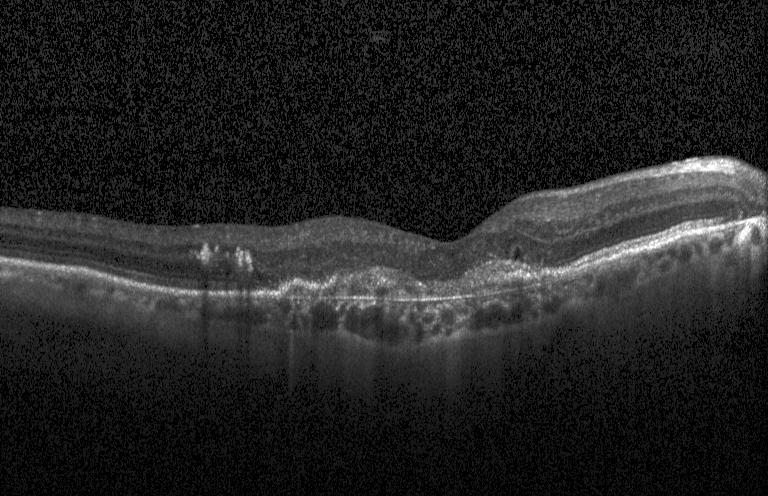
OCT B-scan, spectral-domain OCT.
Macular OCT: a choroidal neovascular membrane.